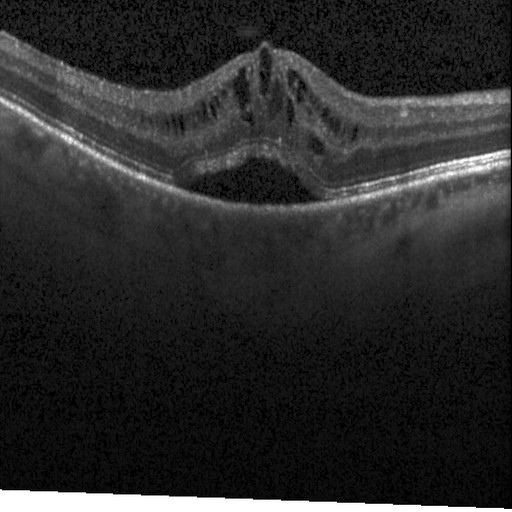 Optical coherence tomography B-scan — Diagnosis: DME.